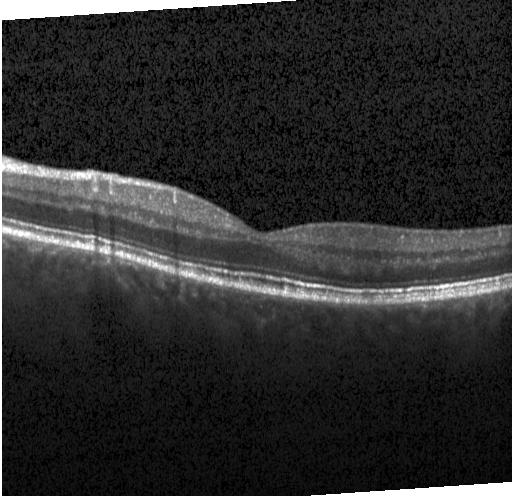

OCT scan showing no CNV, DME, or drusen.